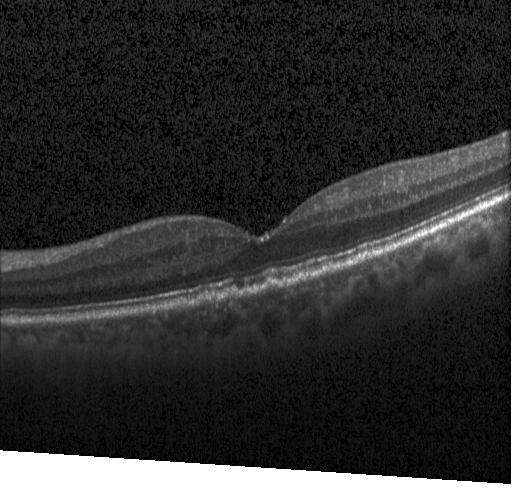 Macular OCT demonstrating sub-RPE drusenoid deposits.